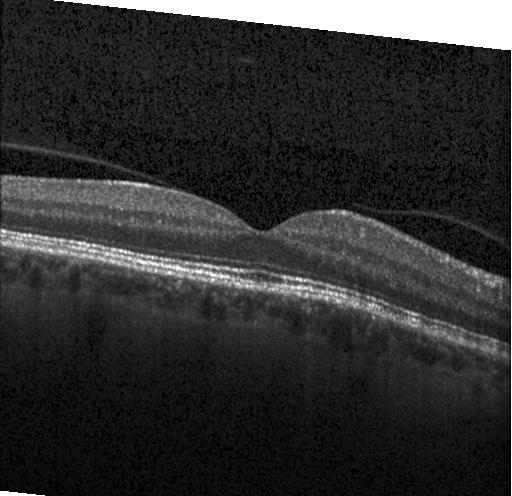
Macular scan, spectral-domain optical coherence tomography, optical coherence tomography B-scan — This B-scan demonstrates no evidence of CNV, DME, or drusen.